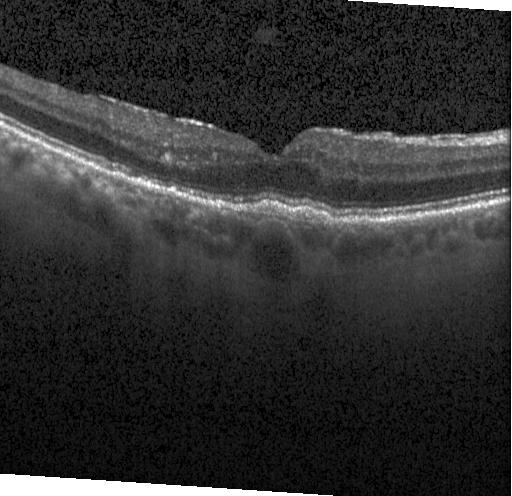
Assessment: a choroidal neovascular membrane.